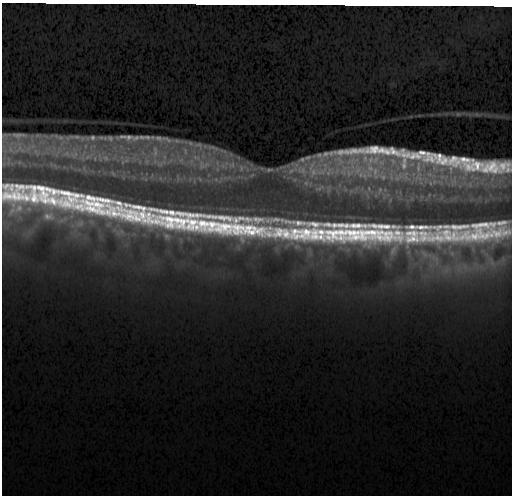
Retinal OCT cross-section. Heidelberg Spectralis OCT system. Macular scan — Finding: neither CNV, DME, nor drusen.